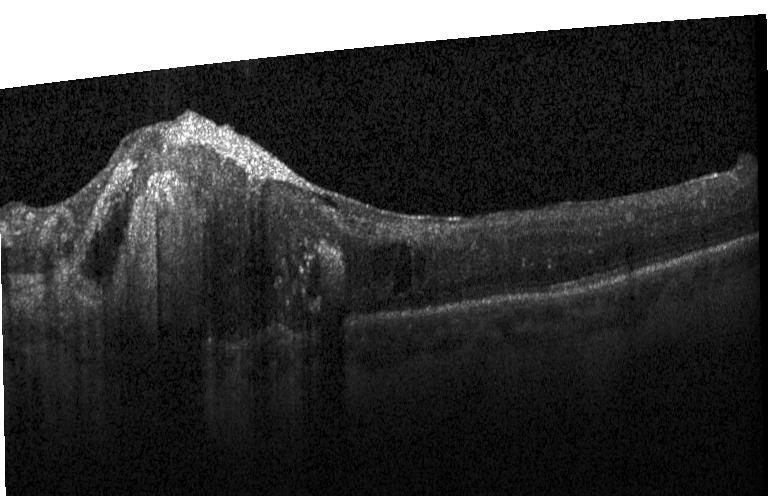
Dx: CNV.